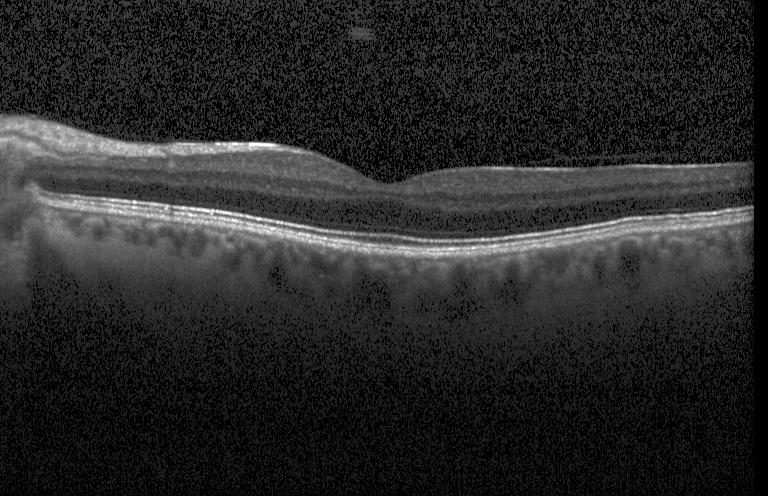
Optical coherence tomography B-scan — Impression: no evidence of choroidal neovascularization, diabetic macular edema, or drusen.